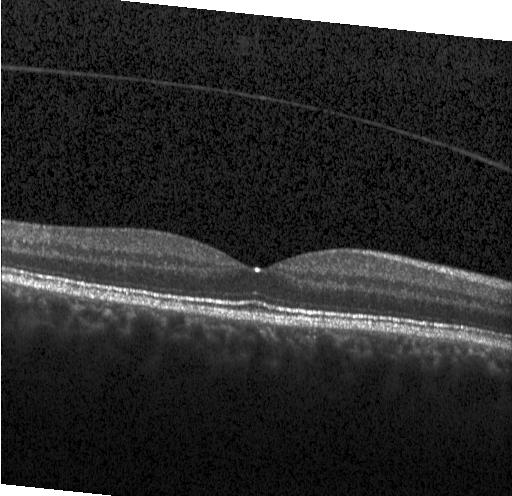

Spectral-domain optical coherence tomography. Optical coherence tomography scan. Centered on the fovea. Acquired on a Heidelberg Spectralis
Macular OCT: no evidence of CNV, DME, or drusen.